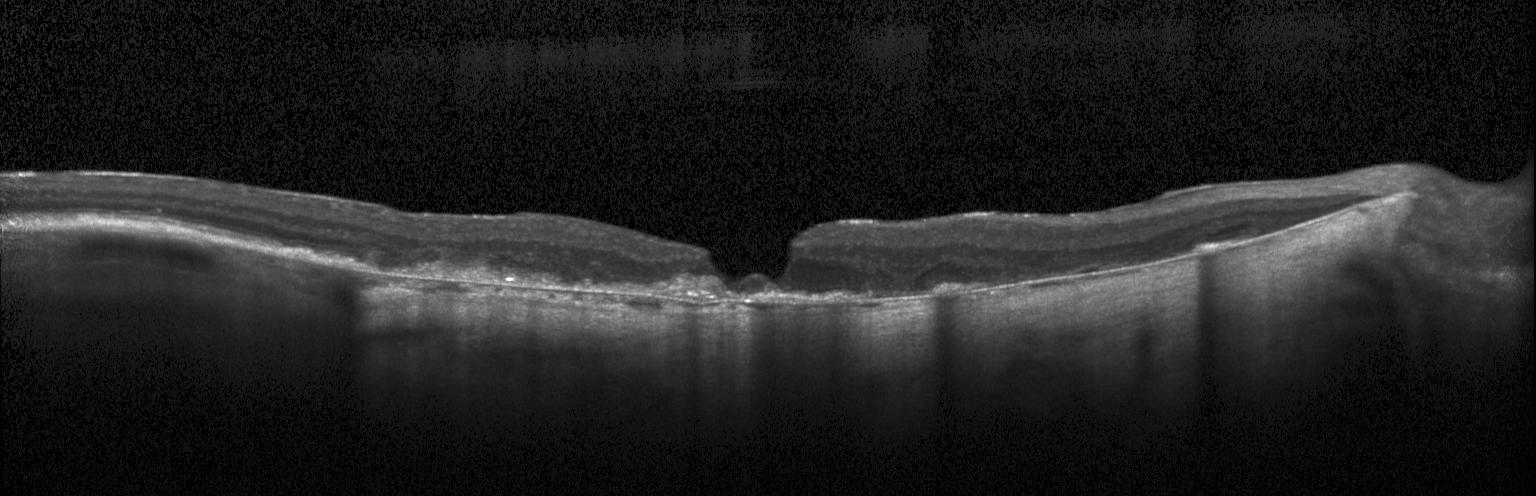

SD-OCT. Heidelberg Spectralis. Retinal OCT cross-section.
A choroidal neovascular membrane.